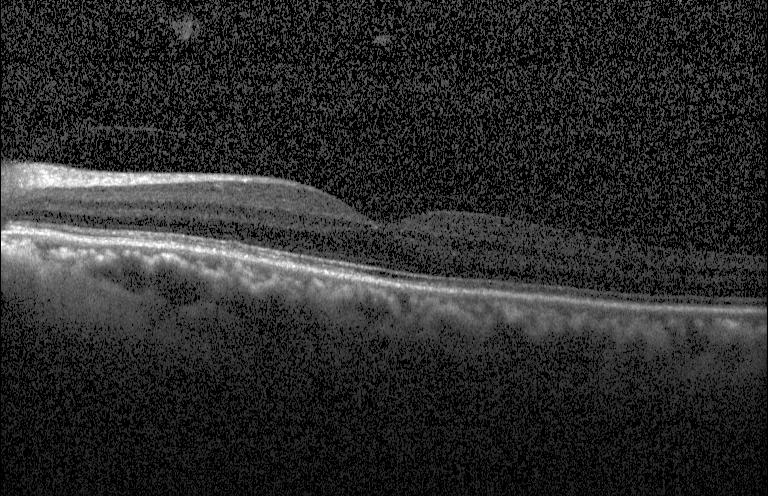
No CNV, DME, or drusen.